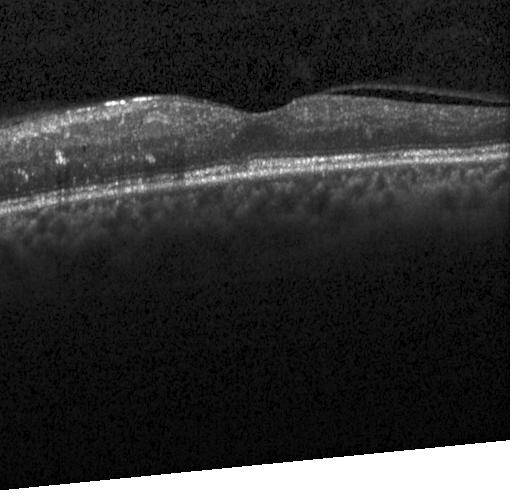
Assessment: DME.